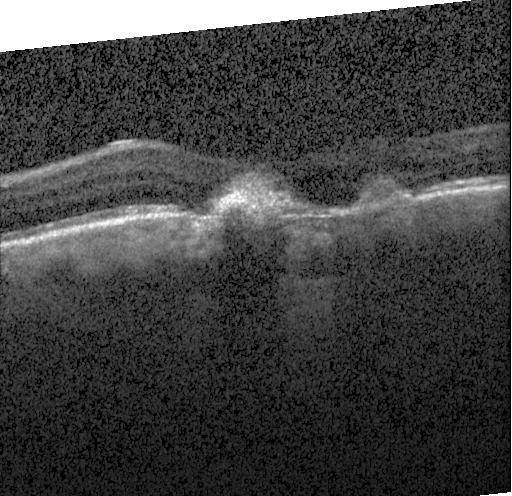 Acquired on a Heidelberg Spectralis · OCT B-scan.
Diagnosis: CNV.